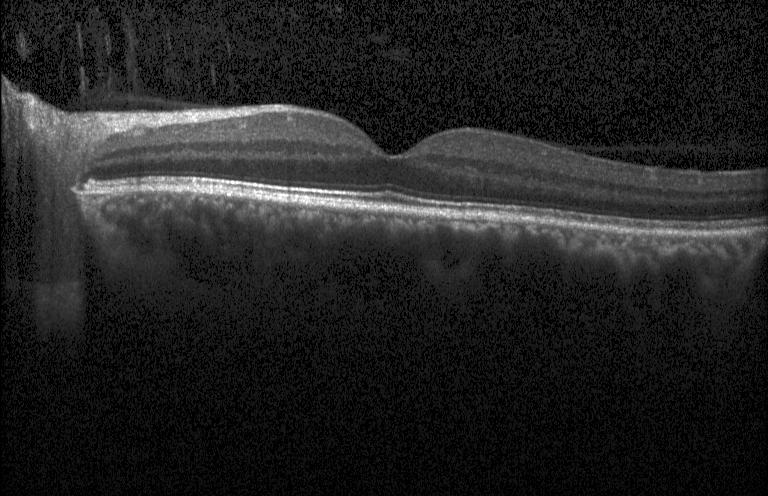

Finding: neither CNV, DME, nor drusen.